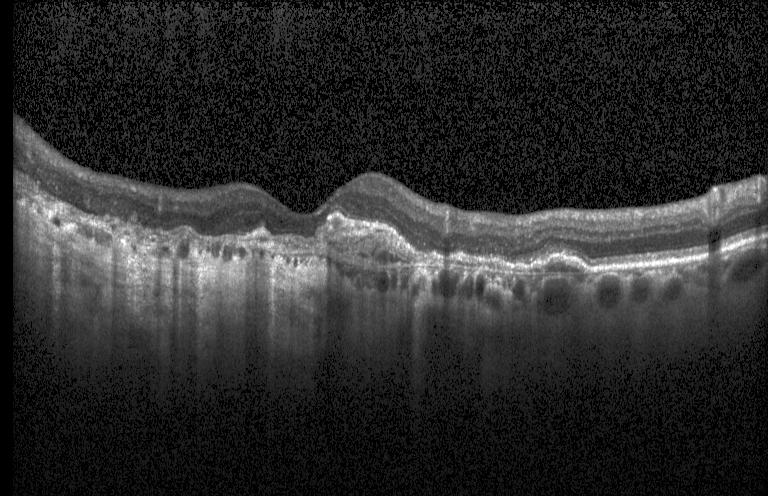 Impression: a choroidal neovascular membrane.